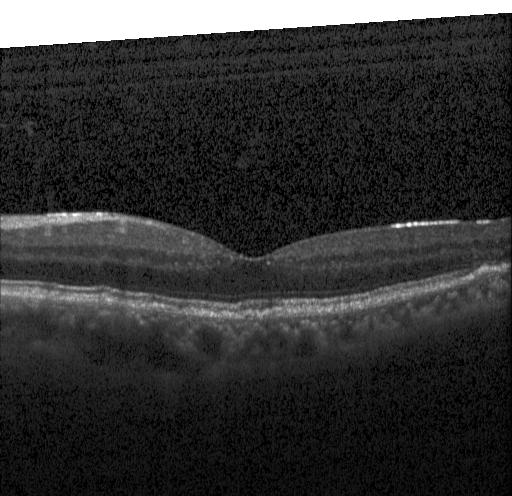

Instrument: Heidelberg Spectralis. Spectral-domain OCT. OCT B-scan
Diagnosis: drusen.